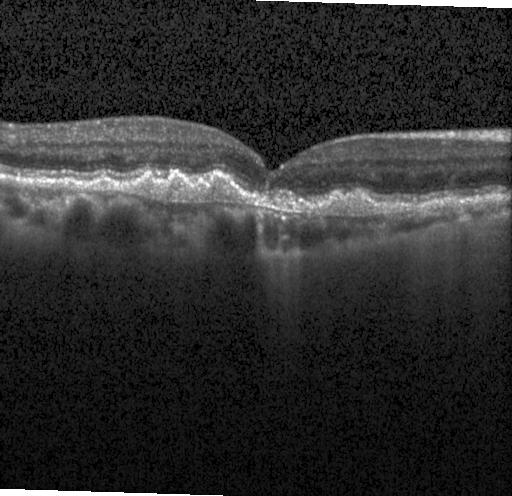
OCT line scan — Assessment: a choroidal neovascular membrane.